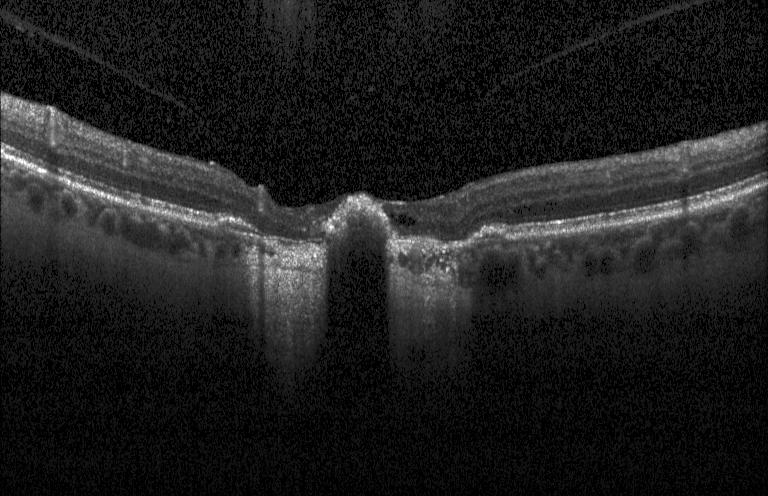 OCT line scan. SD-OCT. Acquired on a Heidelberg Spectralis. The scan shows a choroidal neovascular membrane.